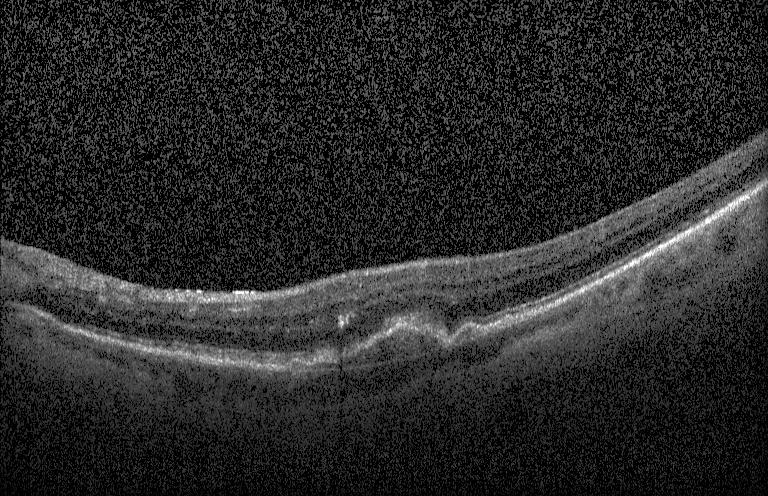 Dx: a choroidal neovascular membrane.